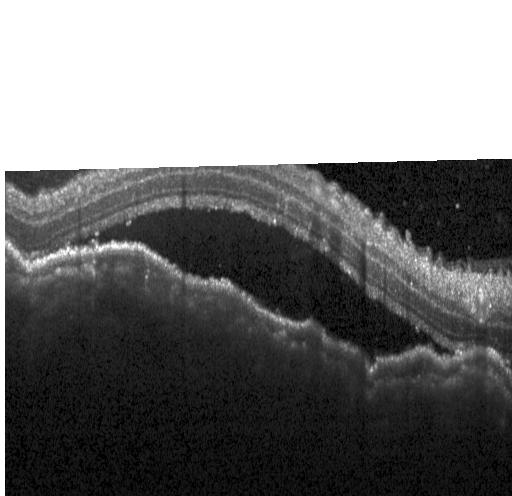
Optical coherence tomography B-scan — The scan shows a choroidal neovascular membrane.